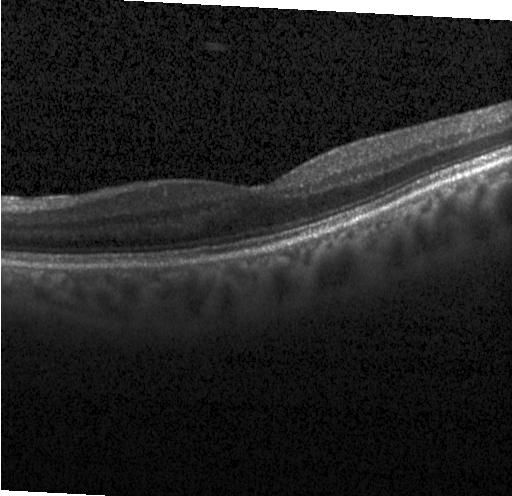
Heidelberg Spectralis; retinal OCT B-scan; horizontal scan through the fovea — Diagnosis: no choroidal neovascularization, diabetic macular edema, or drusen.